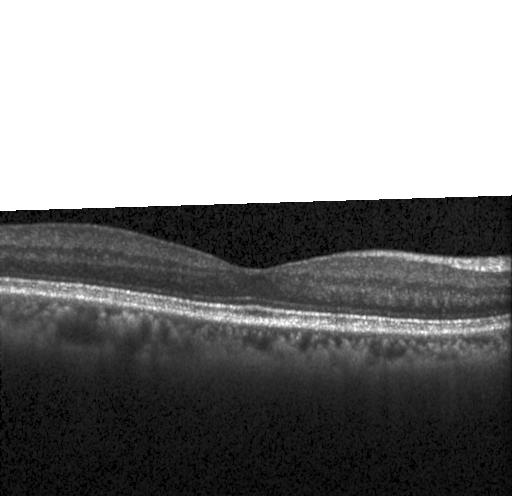

Through the macula, spectral-domain OCT, OCT B-scan — Finding: no CNV, DME, or drusen.